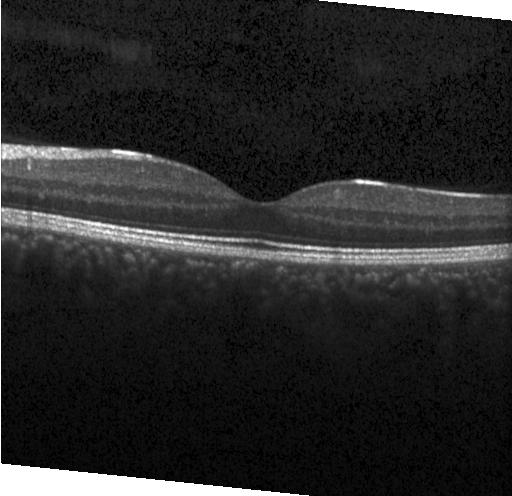 Macular scan. Retinal OCT B-scan. Acquired on a Heidelberg Spectralis. Diagnosis: neither choroidal neovascularization, diabetic macular edema, nor drusen.